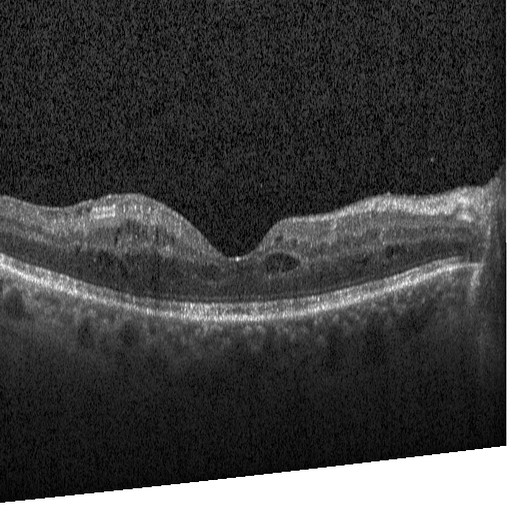 Retinal OCT cross-section — Assessment: diabetic macular edema (DME).